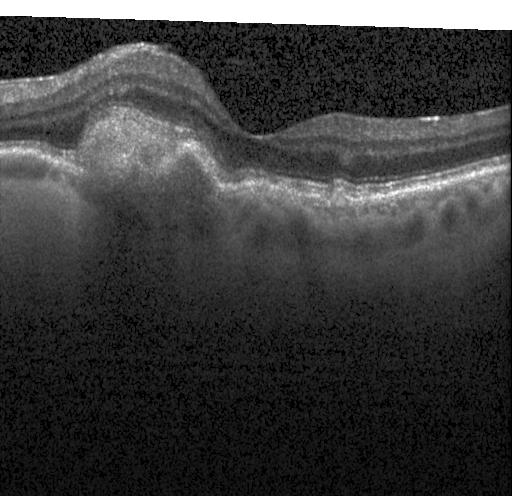
Finding: CNV.